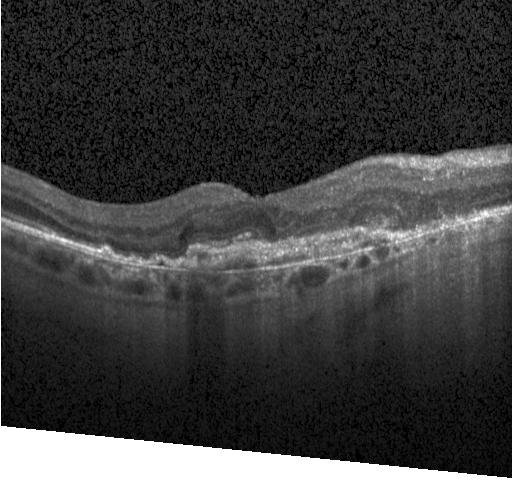

Instrument: Heidelberg Spectralis · retinal OCT B-scan
Diagnosis: a choroidal neovascular membrane.